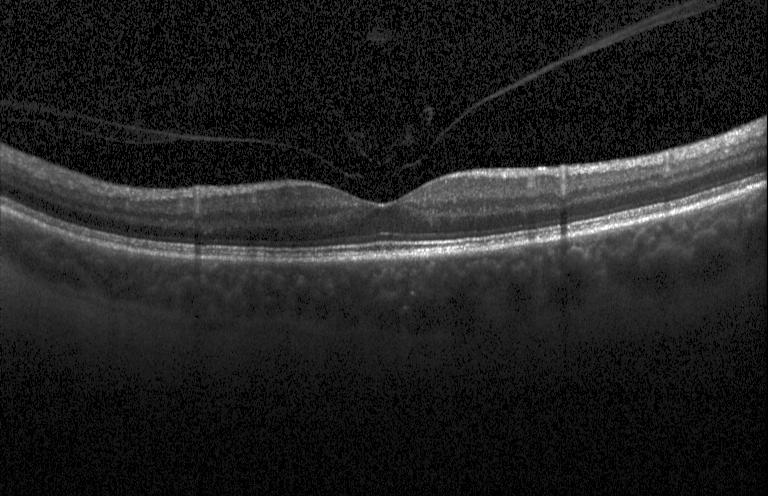

OCT finding: no CNV, DME, or drusen.